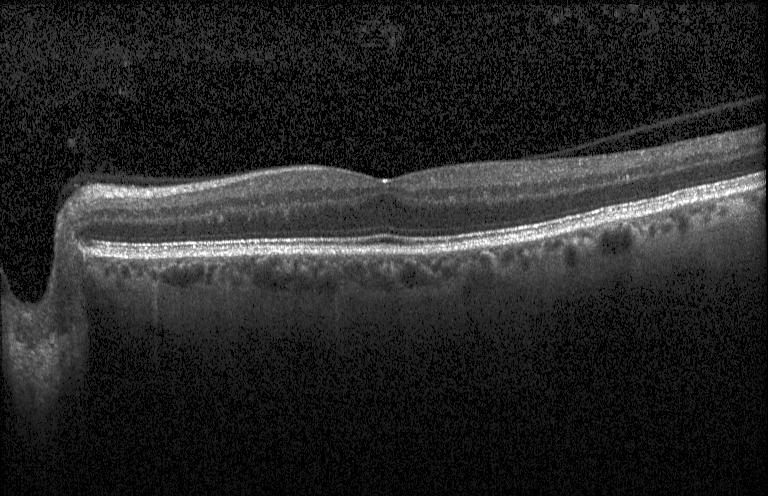

Fovea-centered. OCT B-scan — This B-scan demonstrates neither CNV, DME, nor drusen.